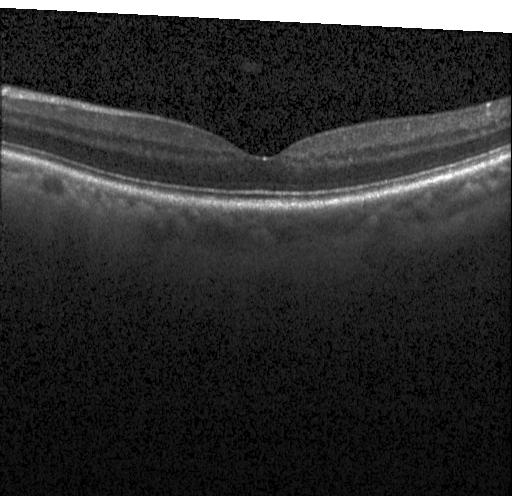
Macular OCT demonstrating neither choroidal neovascularization, diabetic macular edema, nor drusen.